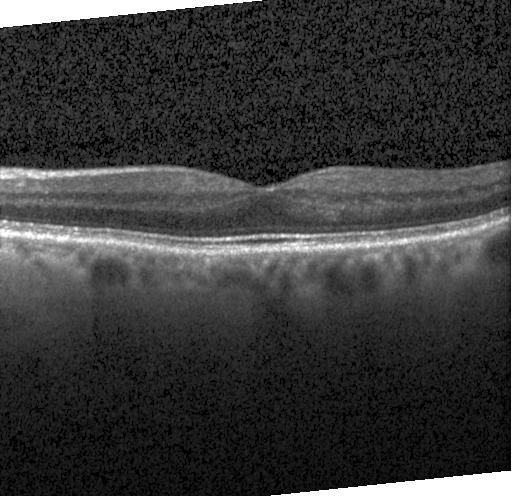

Retinal OCT B-scan. Impression: no evidence of CNV, DME, or drusen.